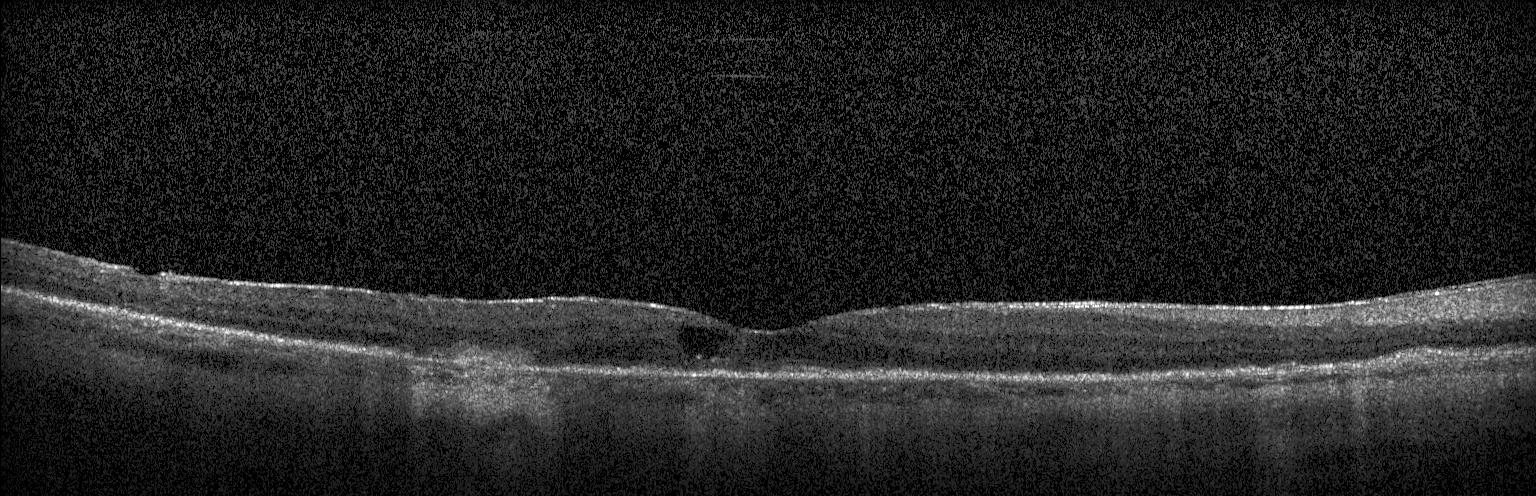

Acquired on a Heidelberg Spectralis, spectral-domain OCT, optical coherence tomography scan. Impression: choroidal neovascularization (CNV).